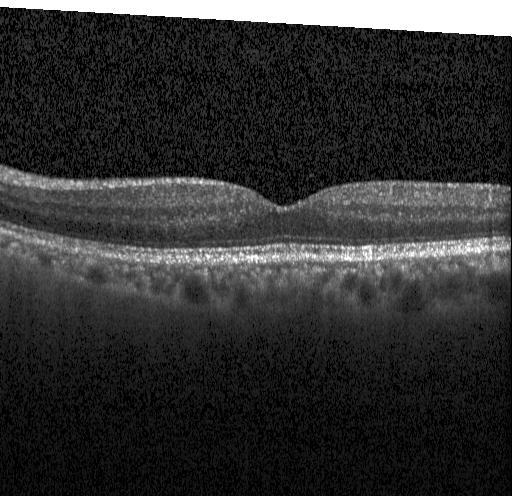
OCT line scan. Diagnosis: neither CNV, DME, nor drusen.